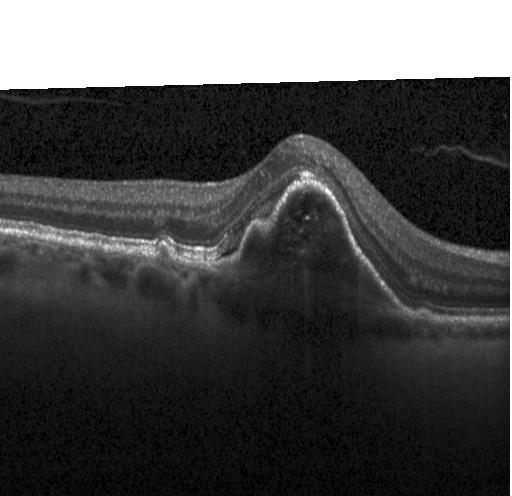

Acquired on a Heidelberg Spectralis · centered on the fovea · OCT B-scan. Diagnosis: CNV.